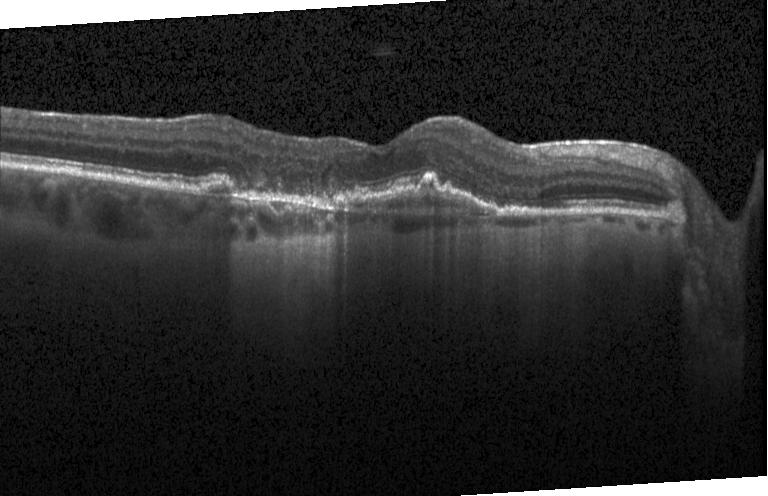

Acquired on a Heidelberg Spectralis; fovea-centered; OCT line scan; spectral-domain OCT
Diagnosis: choroidal neovascularization (CNV).